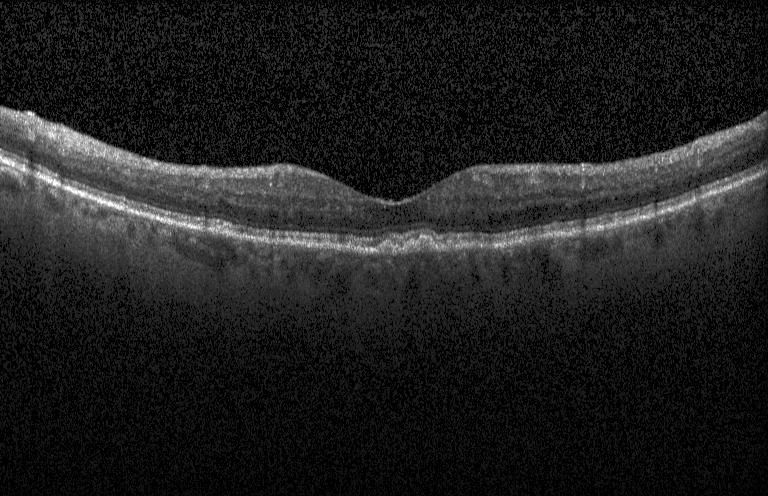

Impression: multiple drusen.